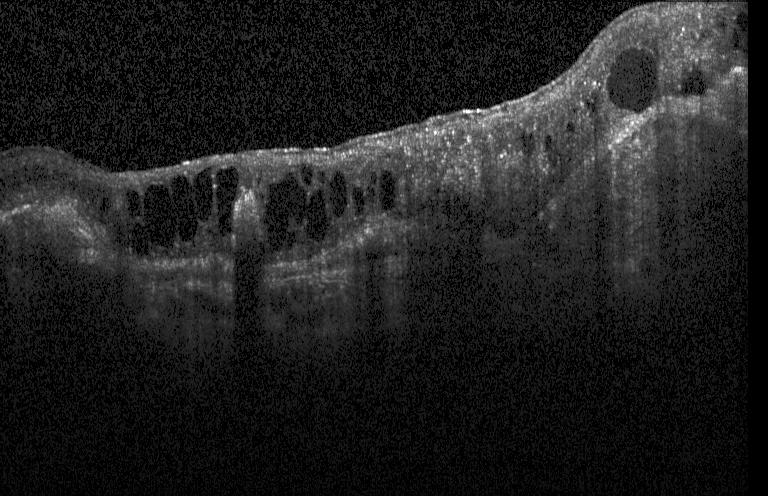

Spectral-domain OCT B-scan: CNV.